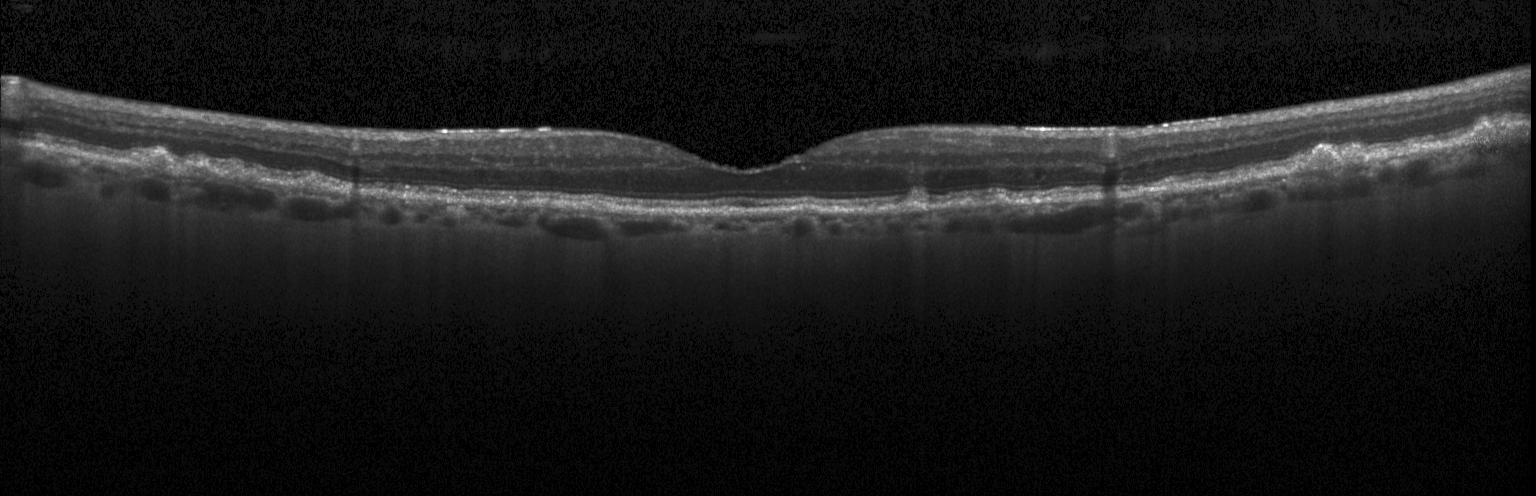 OCT B-scan, fovea-centered — Finding: sub-RPE drusenoid deposits.